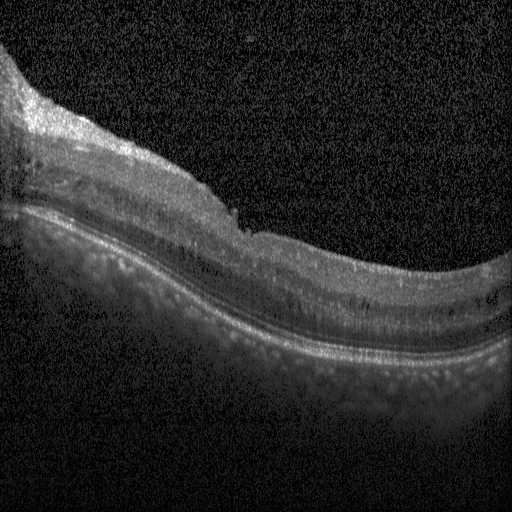

Heidelberg Spectralis OCT system; OCT line scan
This B-scan demonstrates diabetic macular edema (DME).